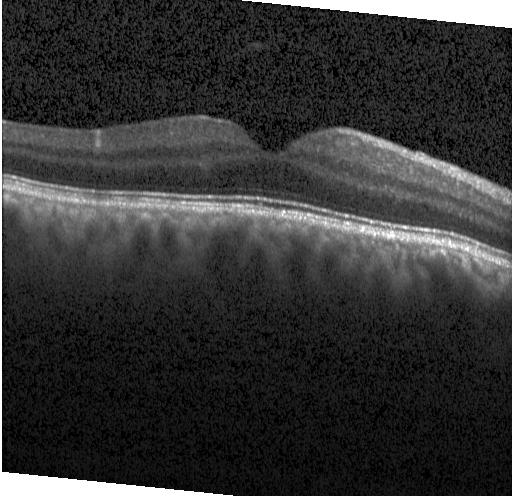 SD-OCT, optical coherence tomography B-scan, Heidelberg Spectralis OCT system, centered on the fovea.
Diagnosis: no choroidal neovascularization, diabetic macular edema, or drusen.